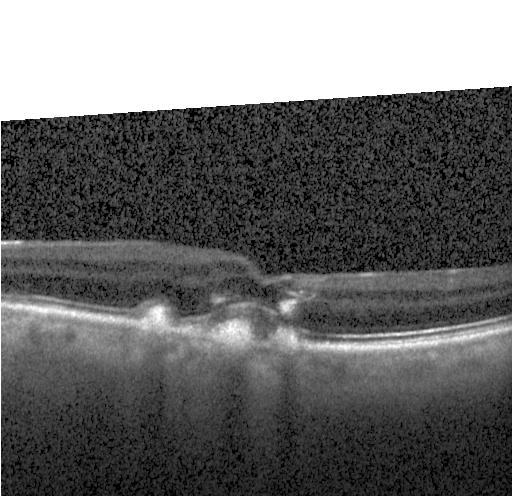 Finding: choroidal neovascularization.